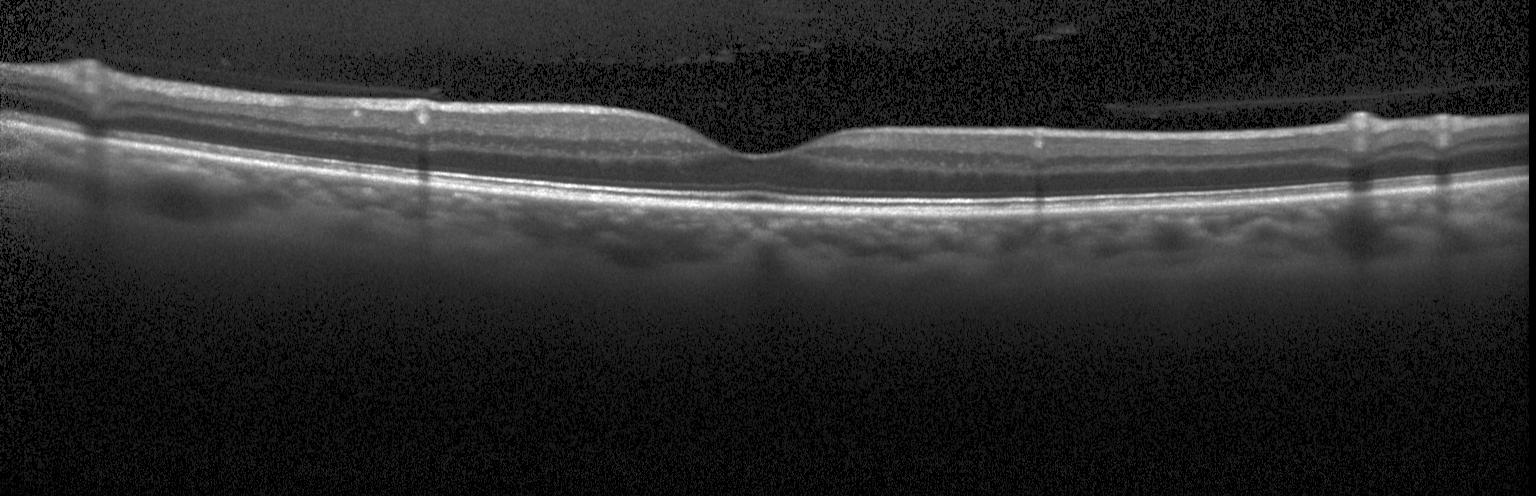
Horizontal scan through the fovea; spectral-domain optical coherence tomography; optical coherence tomography B-scan; Heidelberg Spectralis. Macular OCT: no choroidal neovascularization, diabetic macular edema, or drusen.